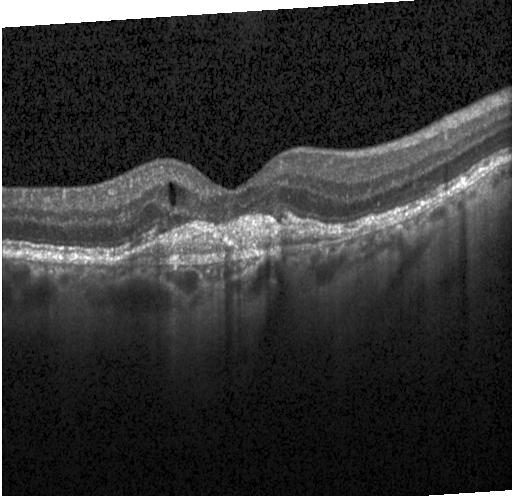 Dx: a choroidal neovascular membrane.